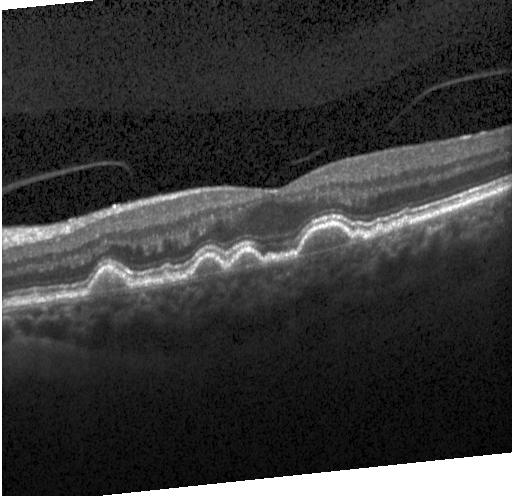

Macular scan · OCT line scan · instrument: Heidelberg Spectralis · spectral-domain optical coherence tomography
Finding: a choroidal neovascular membrane.